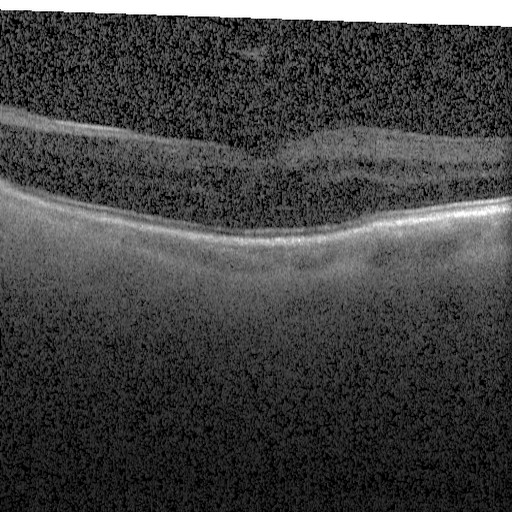 Heidelberg Spectralis OCT system. Optical coherence tomography B-scan
Assessment: DME.